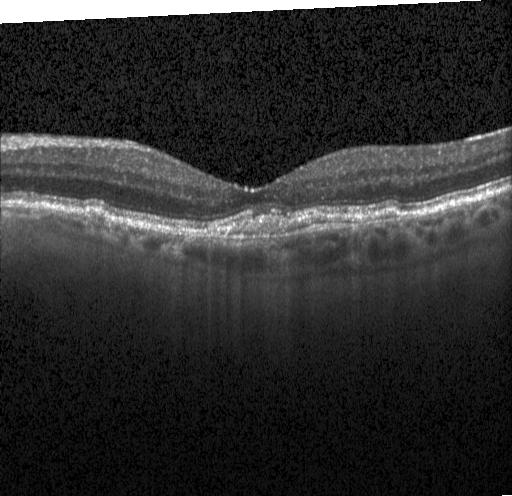
Finding: choroidal neovascularization (CNV).